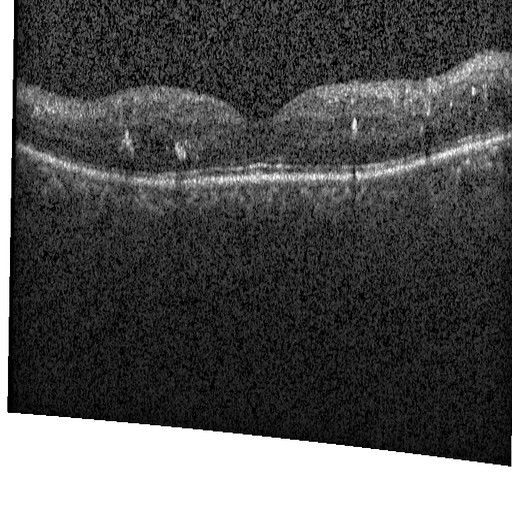 Macular OCT: diabetic macular edema (DME).